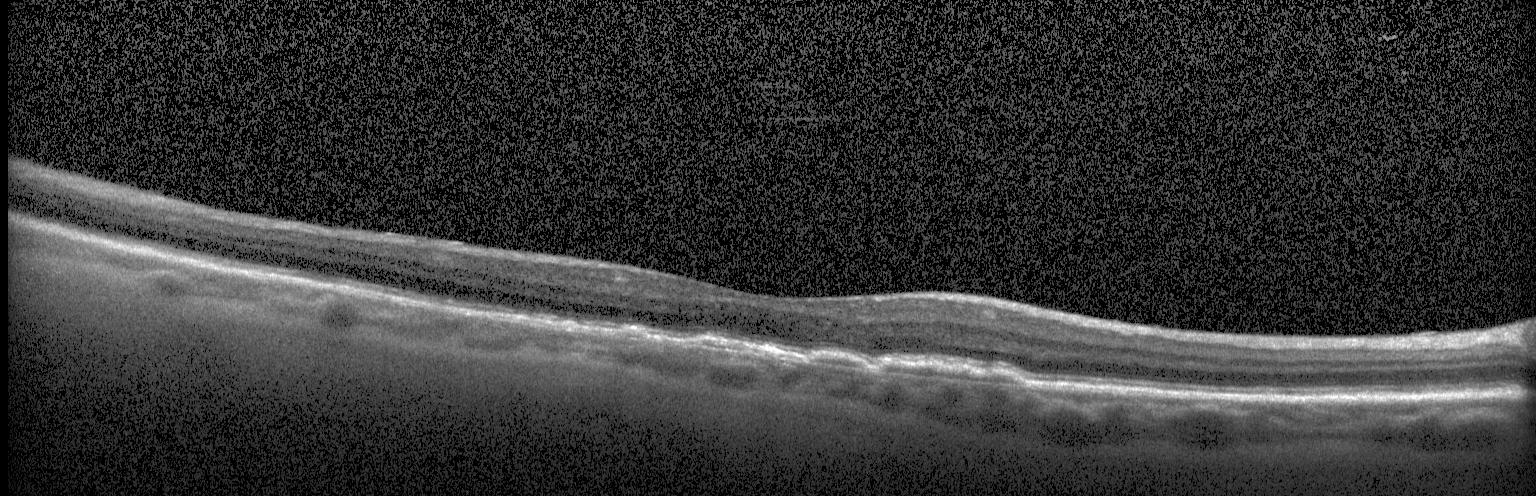

SD-OCT. Acquired on a Heidelberg Spectralis. Optical coherence tomography B-scan. Macular scan.
Dx: a choroidal neovascular membrane.